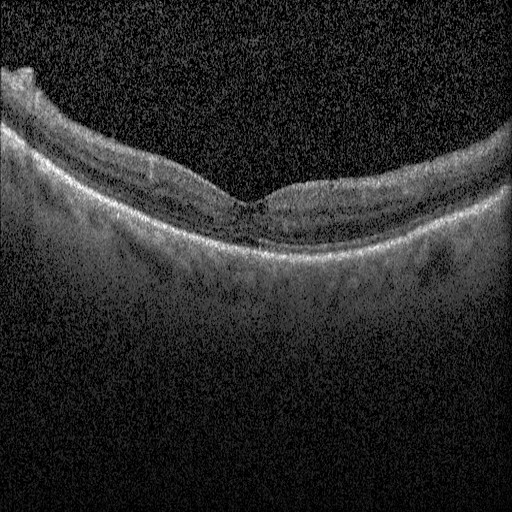
Retinal OCT cross-section. Finding: diabetic macular edema.